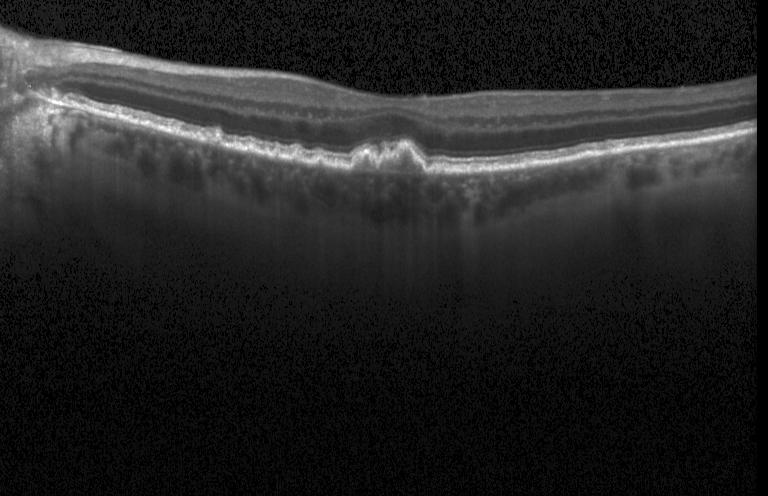
Dx: multiple drusen.